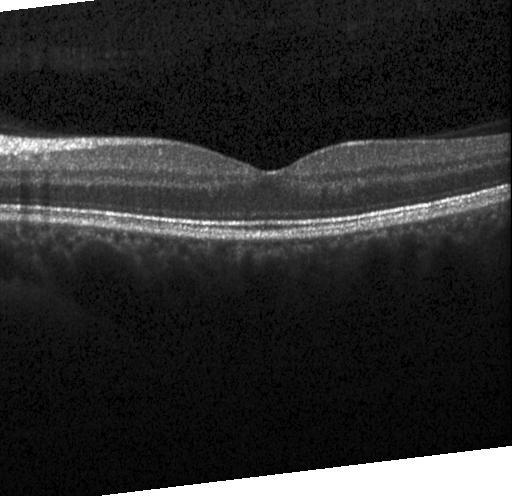

OCT B-scan — Diagnosis: no evidence of CNV, DME, or drusen.